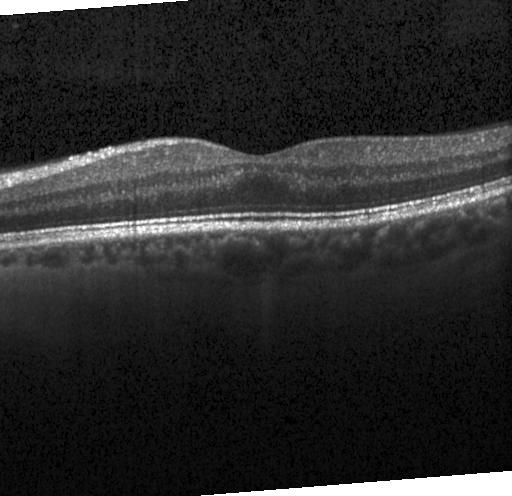 OCT B-scan showing no choroidal neovascularization, no diabetic macular edema, and no drusen.